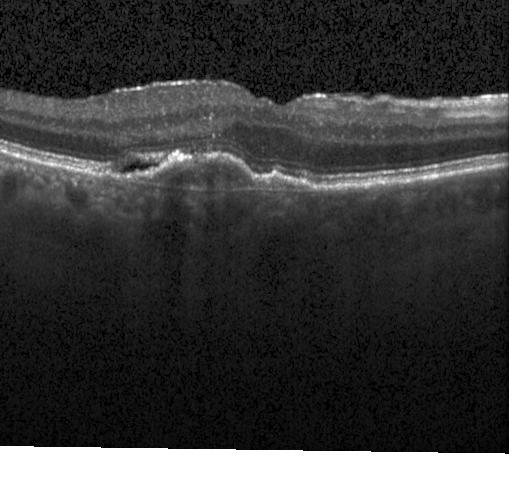

Optical coherence tomography B-scan · Heidelberg Spectralis · fovea-centered · spectral-domain optical coherence tomography.
Finding: choroidal neovascularization.